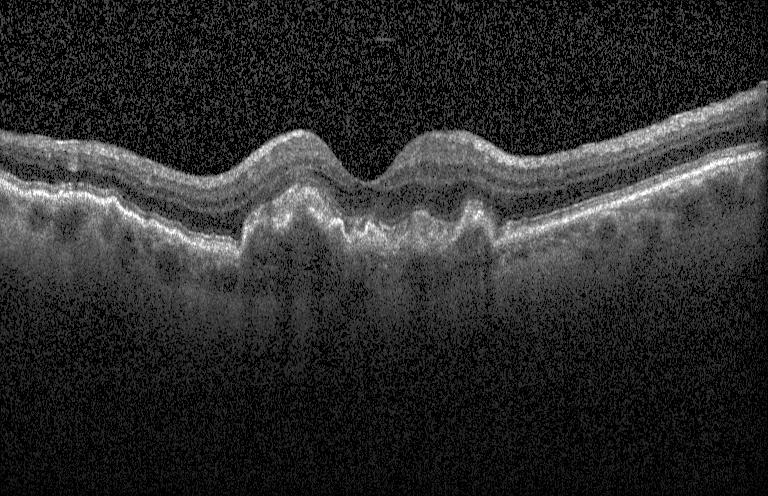

Retinal OCT cross-section
Finding: choroidal neovascularization.